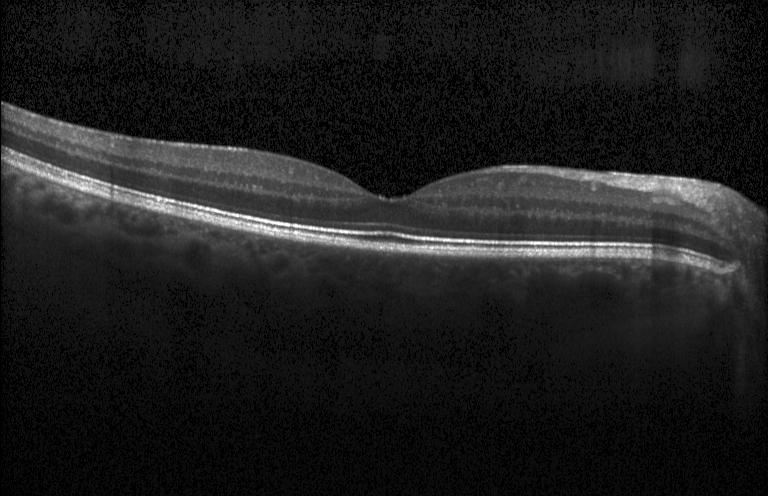
Optical coherence tomography scan · centered on the fovea.
OCT finding: no CNV, no DME, and no drusen.